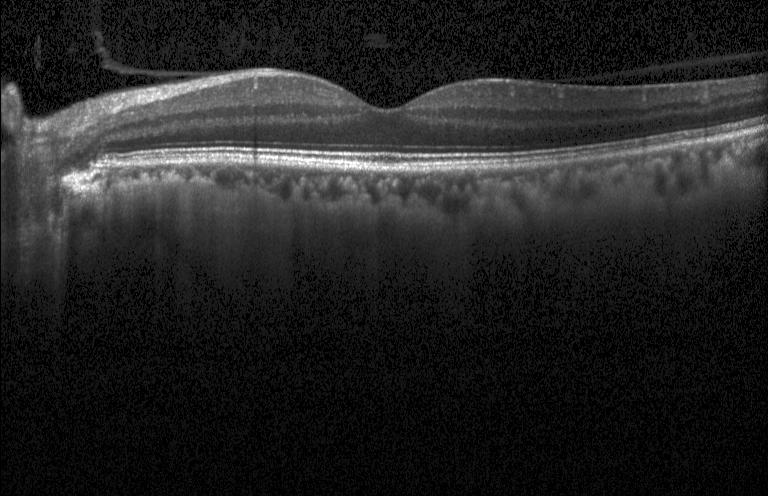

Through the macula; OCT B-scan; Heidelberg Spectralis OCT system.
Impression: no CNV, no DME, and no drusen.